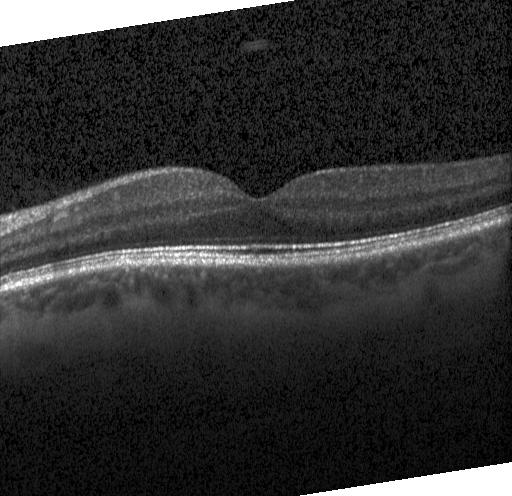

Centered on the fovea; OCT line scan — No CNV, DME, or drusen.